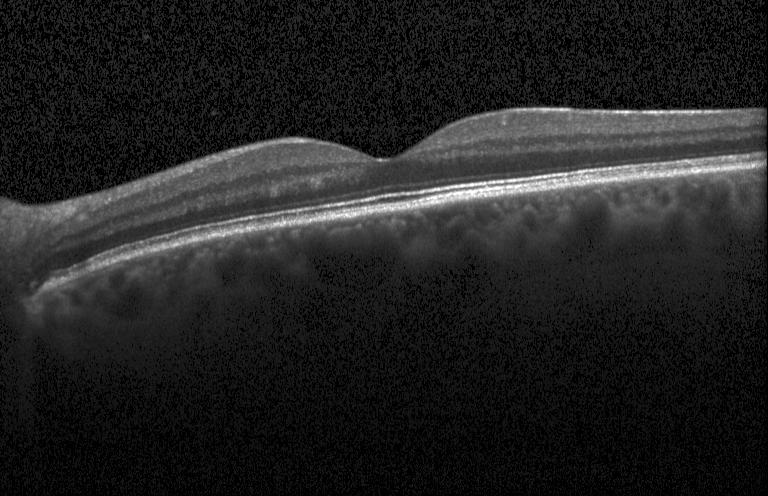
Optical coherence tomography scan. This B-scan demonstrates neither choroidal neovascularization, diabetic macular edema, nor drusen.